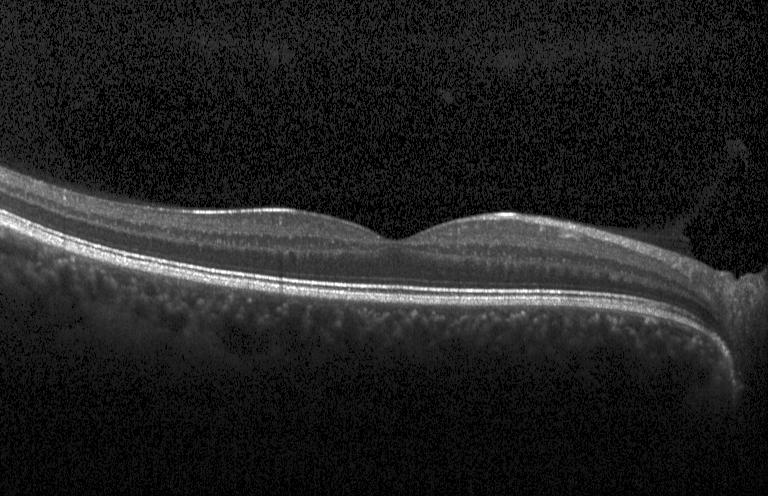
Optical coherence tomography scan.
Dx: no choroidal neovascularization, diabetic macular edema, or drusen.